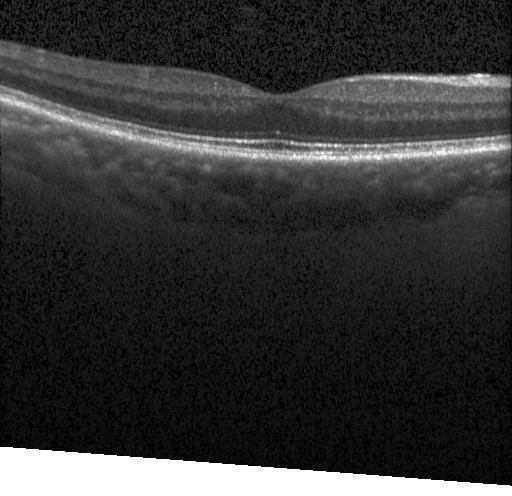

Spectral-domain OCT, optical coherence tomography B-scan. Assessment: no choroidal neovascularization, no diabetic macular edema, and no drusen.